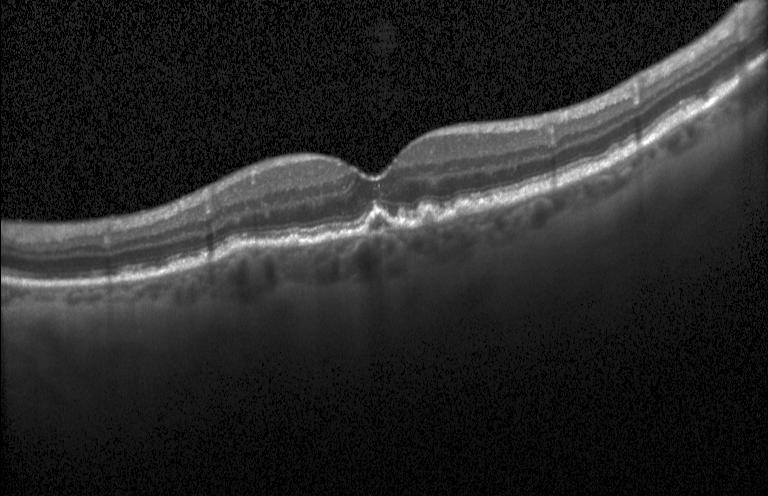

Retinal OCT cross-section
Diagnosis: multiple drusen.